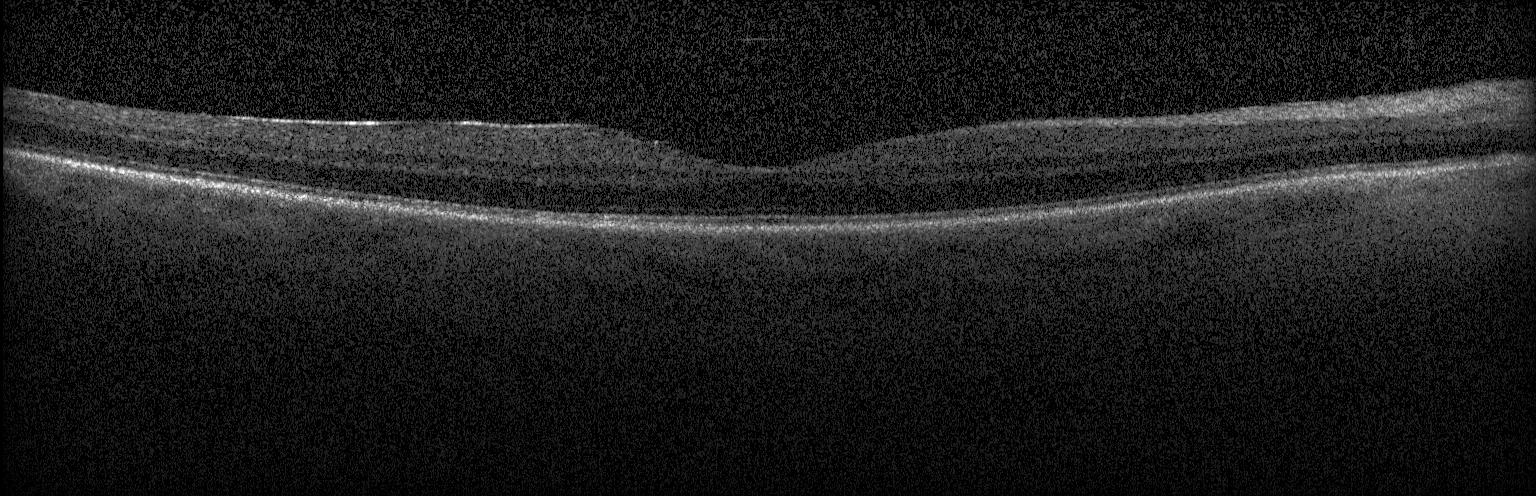
Diagnosis: neither choroidal neovascularization, diabetic macular edema, nor drusen.